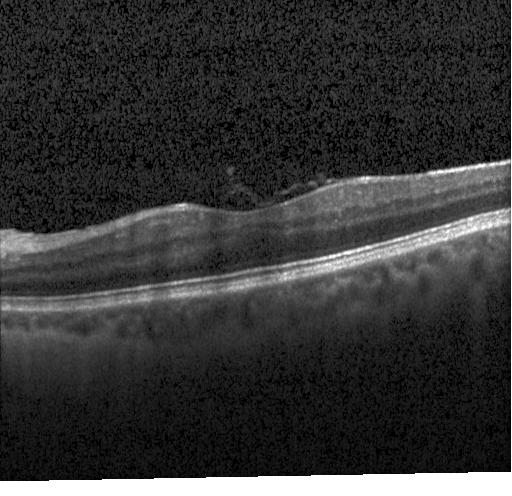
OCT scan showing no CNV, no DME, and no drusen.